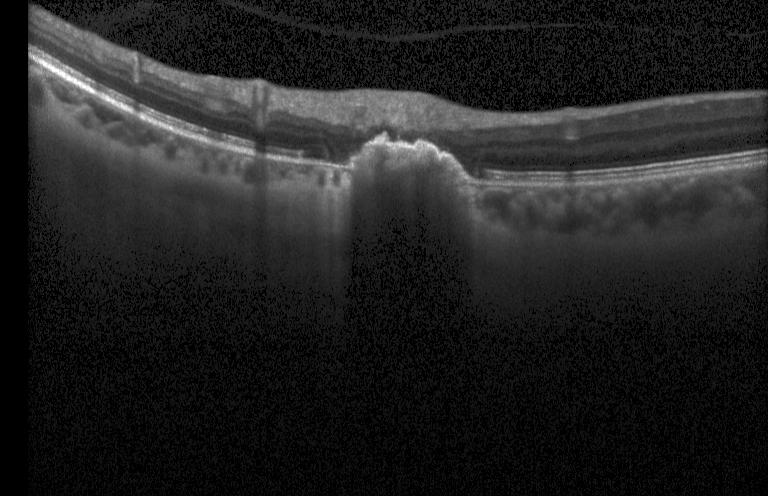
OCT scan showing choroidal neovascularization.